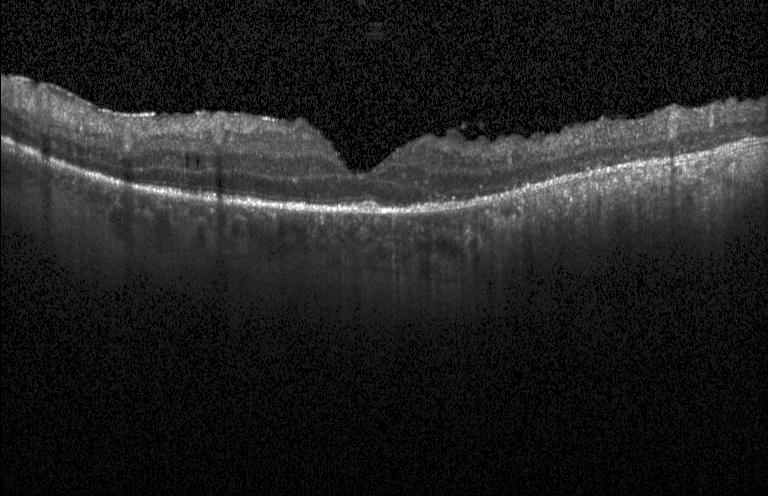 Impression: diabetic macular edema (DME).